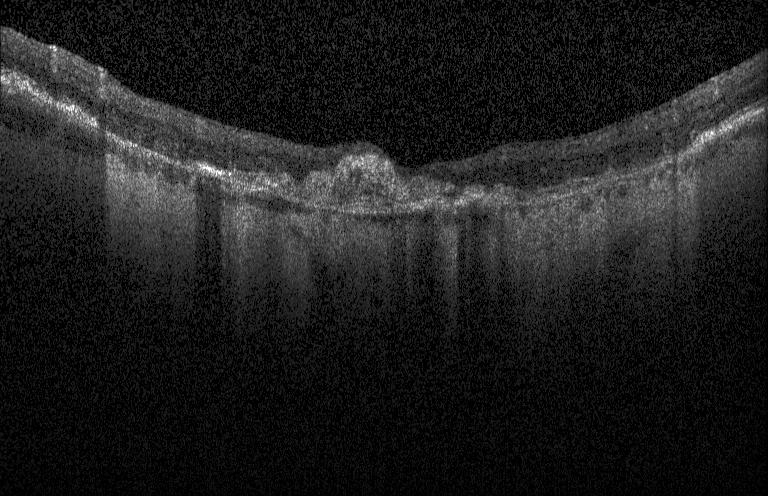
SD-OCT · OCT line scan.
Macular OCT: choroidal neovascularization.